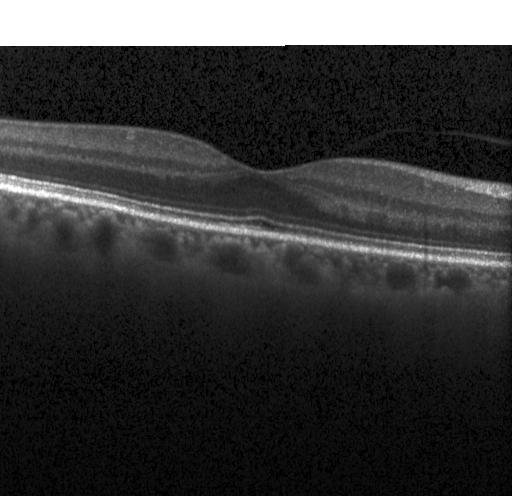

The scan shows no CNV, no DME, and no drusen.